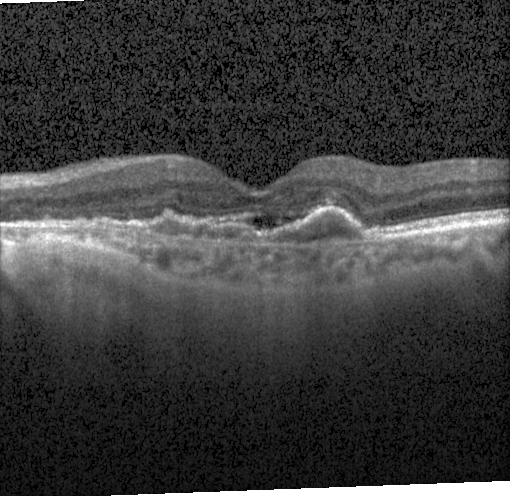 Macular OCT demonstrating choroidal neovascularization.